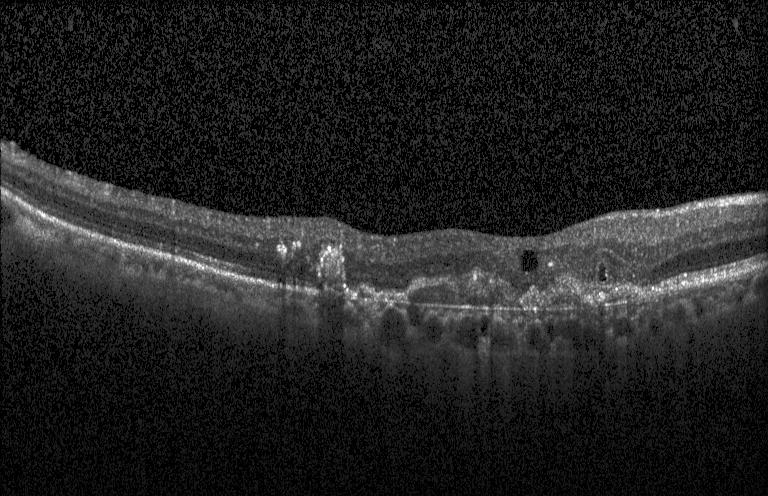
Spectral-domain optical coherence tomography, through the macula, Heidelberg Spectralis, retinal OCT cross-section.
Impression: CNV.